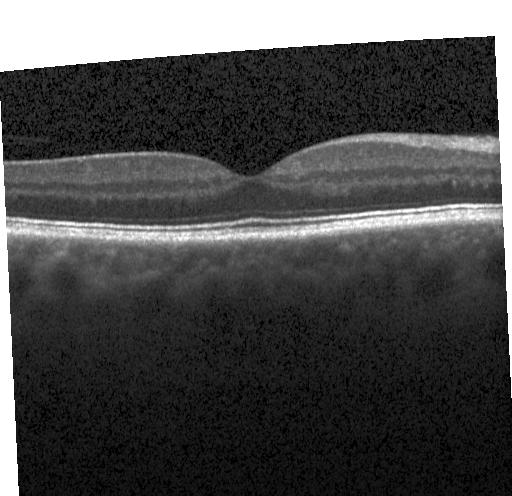
Impression: no choroidal neovascularization, no diabetic macular edema, and no drusen.